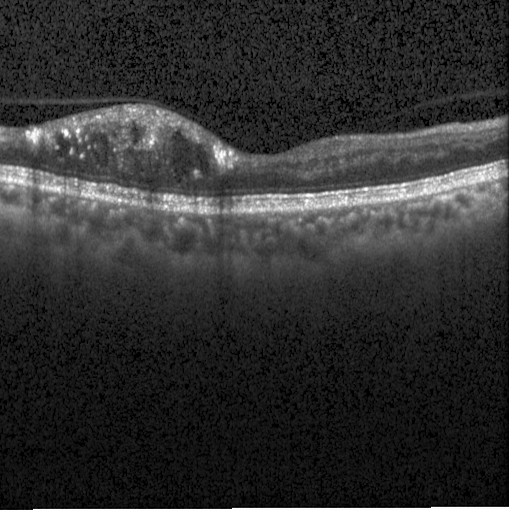 OCT line scan. Spectral-domain optical coherence tomography. Centered on the fovea
Finding: diabetic macular edema.